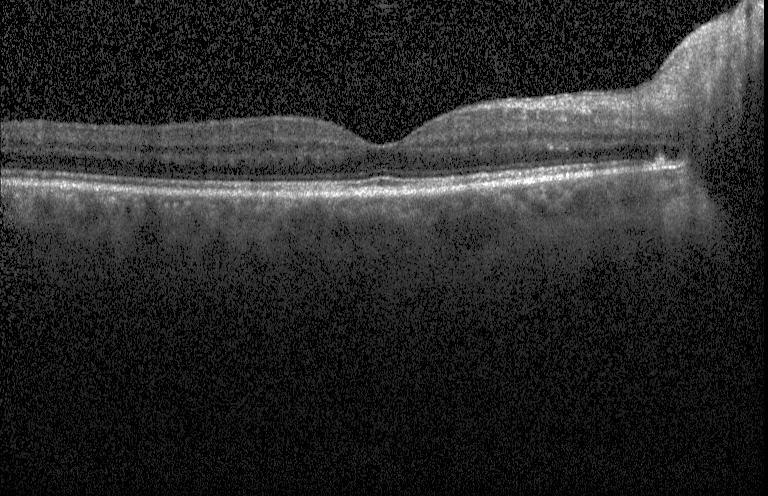 OCT line scan — OCT finding: no evidence of choroidal neovascularization, diabetic macular edema, or drusen.